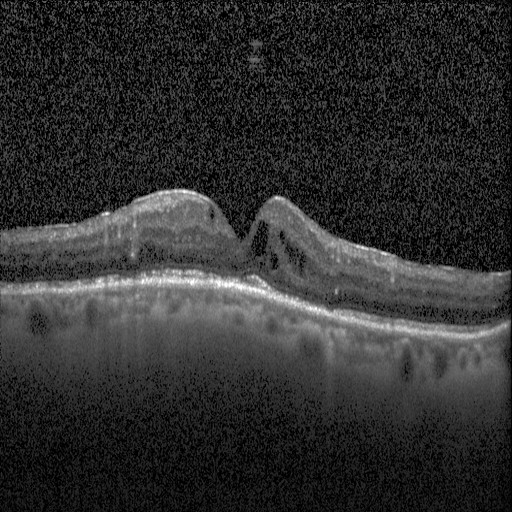 Macular OCT demonstrating diabetic macular edema.